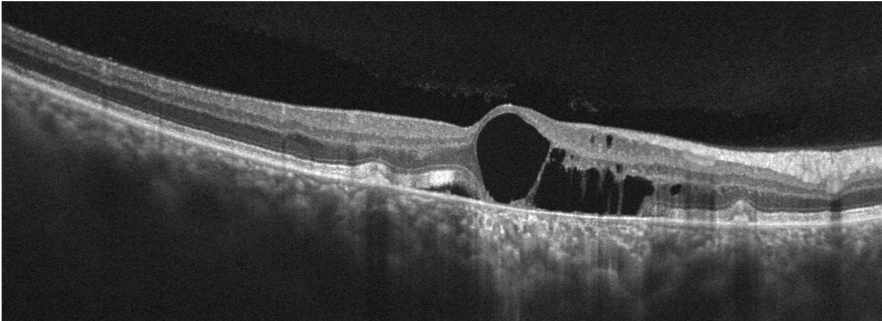
Instrument: Optovue Avanti RTVue XR. Retinal OCT cross-section. Macular scan.
Finding: age-related macular degeneration.